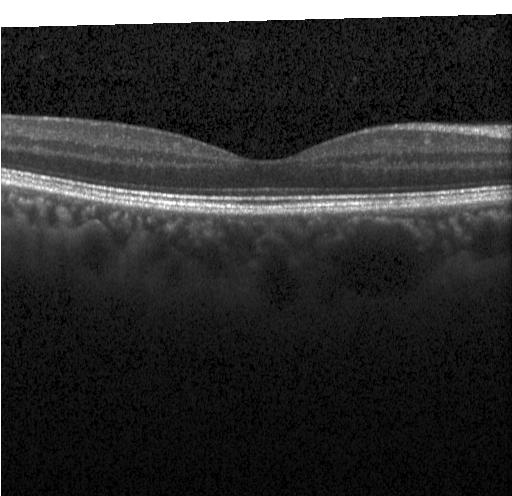
OCT B-scan · instrument: Heidelberg Spectralis. Finding: no evidence of CNV, DME, or drusen.